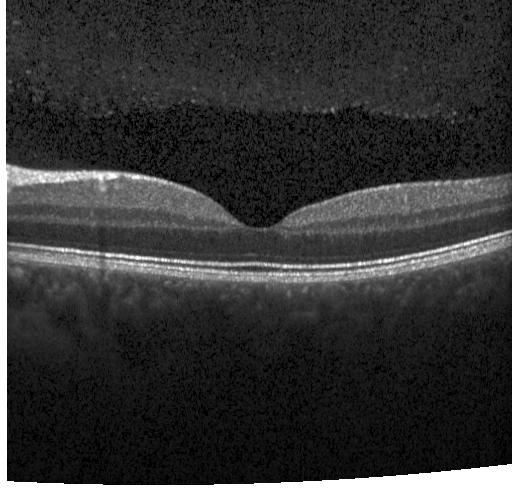
Horizontal scan through the fovea; optical coherence tomography B-scan; SD-OCT; Heidelberg Spectralis. OCT finding: no choroidal neovascularization, diabetic macular edema, or drusen.